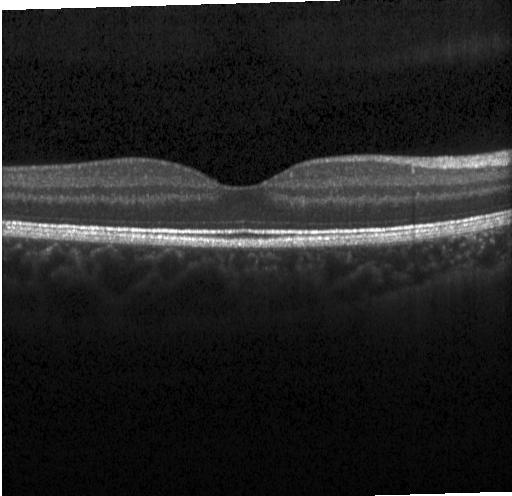
The scan shows no choroidal neovascularization, diabetic macular edema, or drusen.